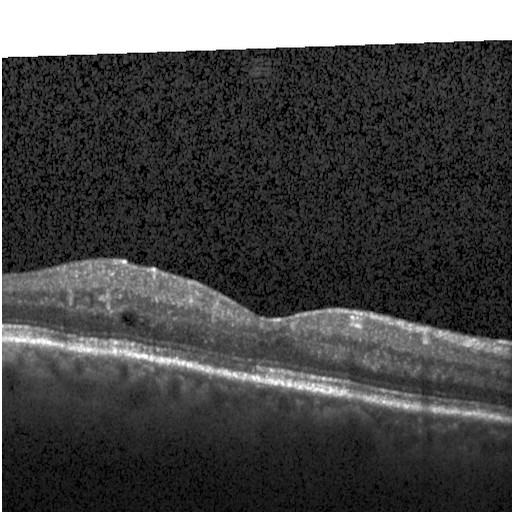
Instrument: Heidelberg Spectralis · optical coherence tomography B-scan
Impression: diabetic macular edema (DME).